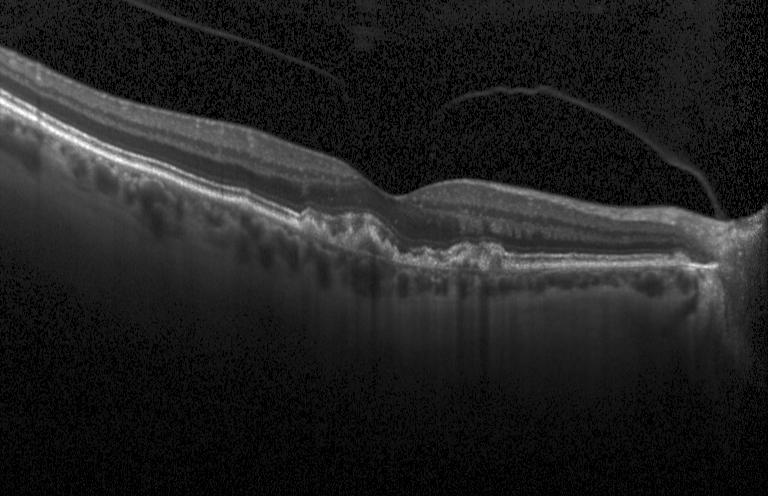

This B-scan demonstrates a choroidal neovascular membrane.